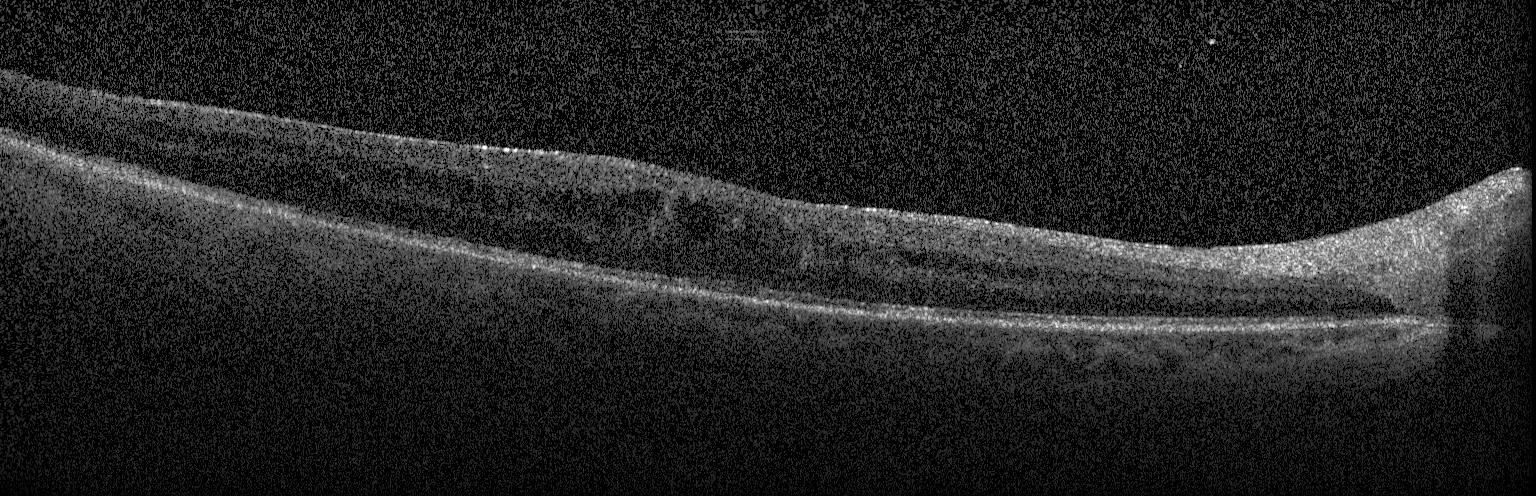

Macular OCT demonstrating DME.